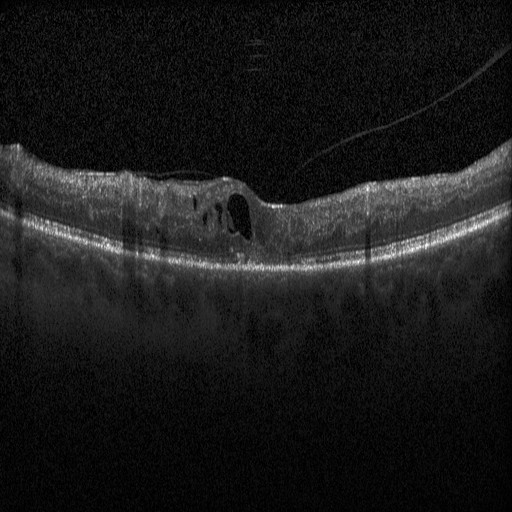 OCT B-scan; macular scan; Heidelberg Spectralis OCT system
DME.